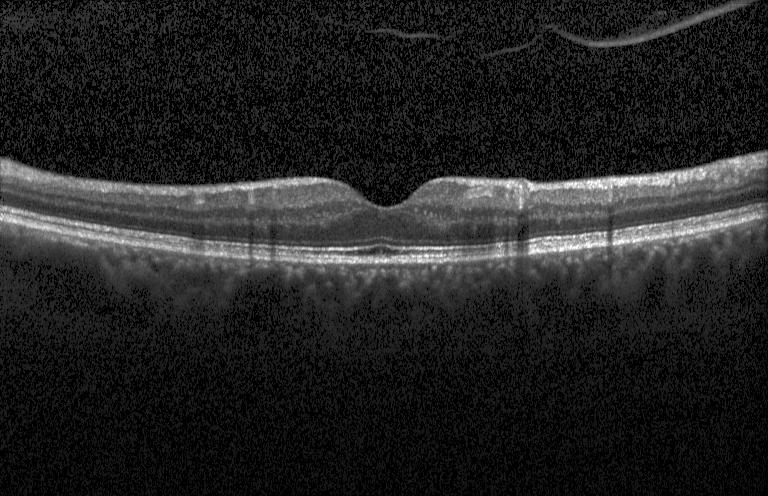
OCT line scan, spectral-domain optical coherence tomography. Diagnosis: no choroidal neovascularization, diabetic macular edema, or drusen.